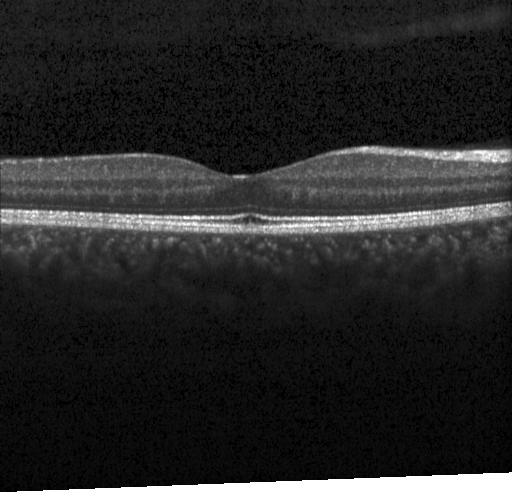 Macular OCT: no choroidal neovascularization, no diabetic macular edema, and no drusen.